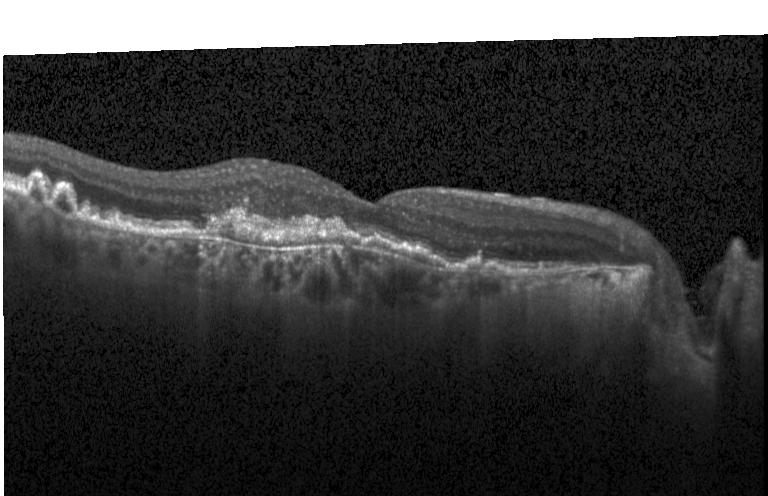 Centered on the fovea, retinal OCT B-scan
Impression: a choroidal neovascular membrane.